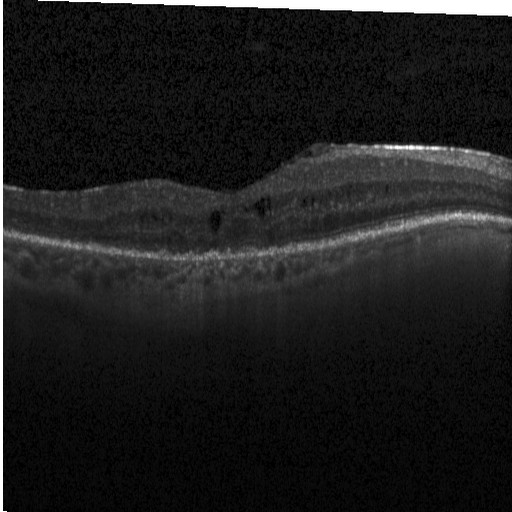 Assessment: DME.